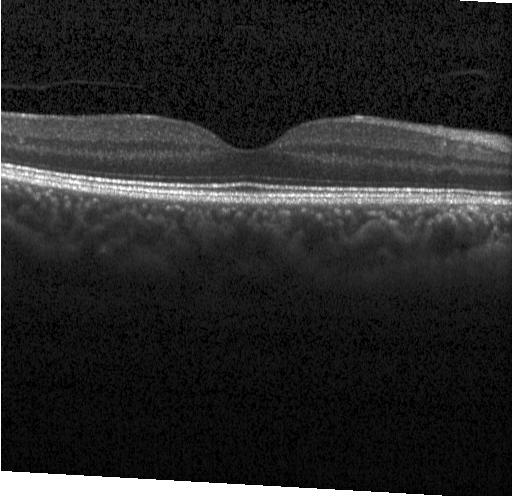 Optical coherence tomography scan. Impression: no CNV, no DME, and no drusen.